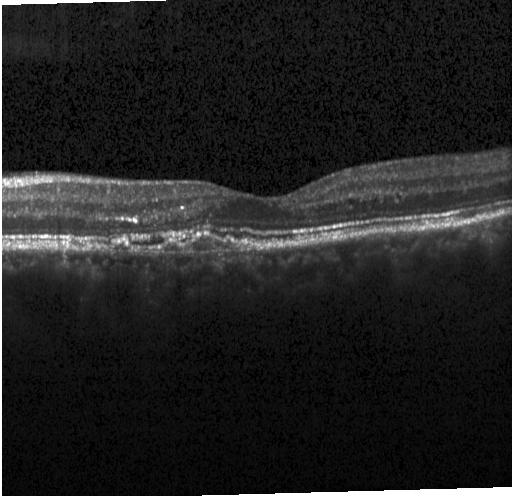
Heidelberg Spectralis. Macular scan. Optical coherence tomography B-scan. SD-OCT — Diagnosis: CNV.